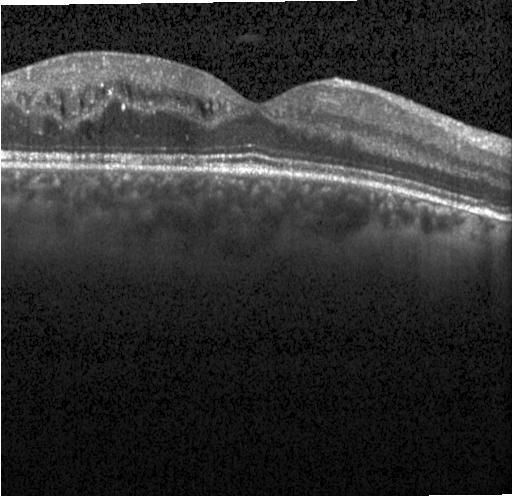
Finding: DME.